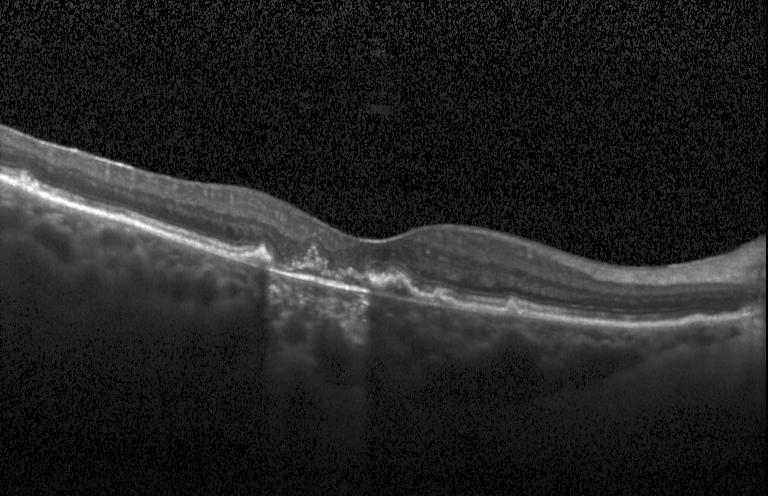

Heidelberg Spectralis OCT system · OCT line scan · horizontal scan through the fovea. Diagnosis: choroidal neovascularization.